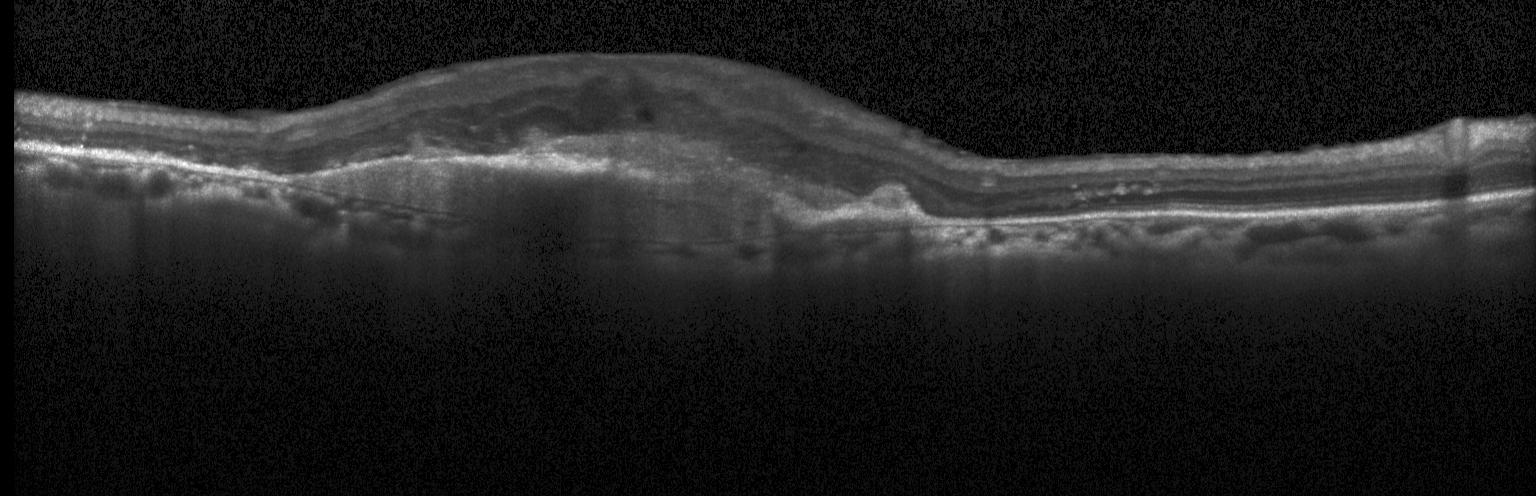
OCT B-scan — Assessment: a choroidal neovascular membrane.